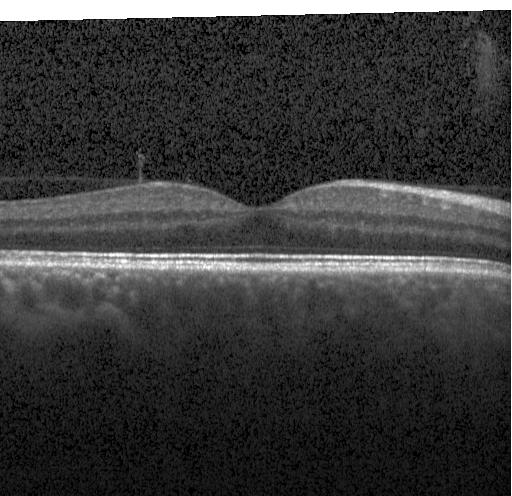 This B-scan demonstrates no evidence of CNV, DME, or drusen.